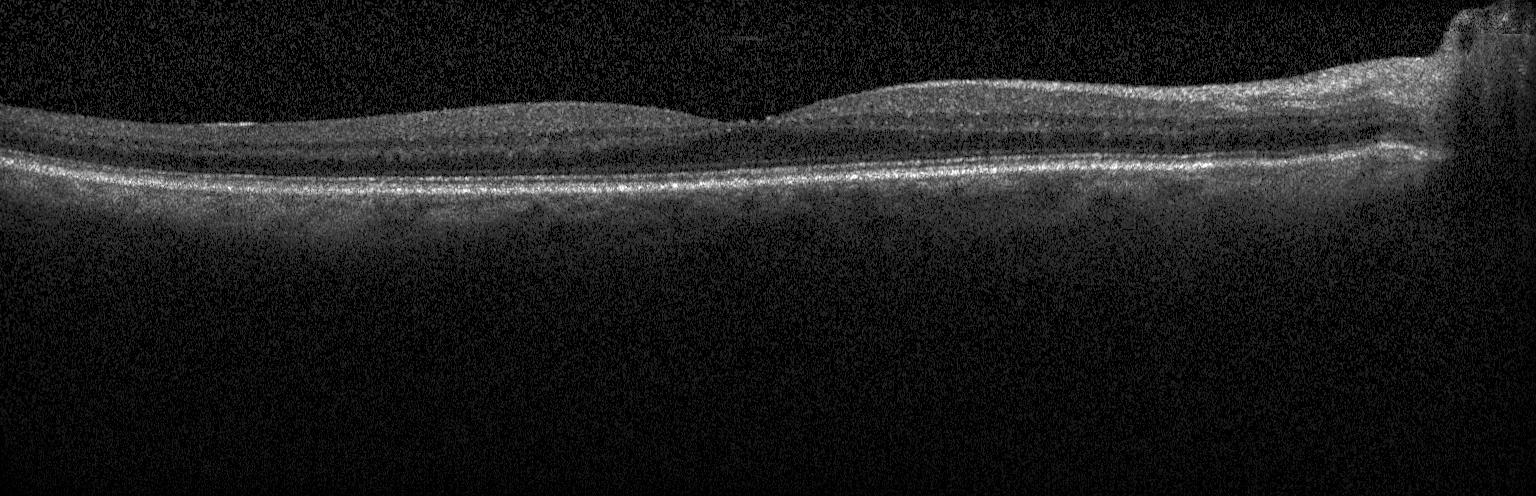
Spectral-domain optical coherence tomography. Optical coherence tomography scan. Horizontal scan through the fovea. Heidelberg Spectralis OCT system. Diagnosis: neither choroidal neovascularization, diabetic macular edema, nor drusen.